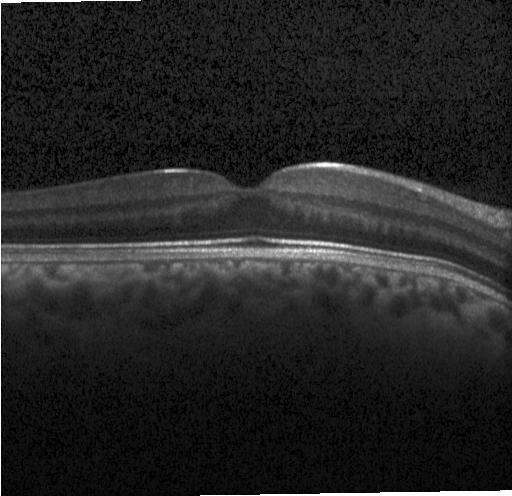

Retinal OCT cross-section showing no choroidal neovascularization, diabetic macular edema, or drusen.